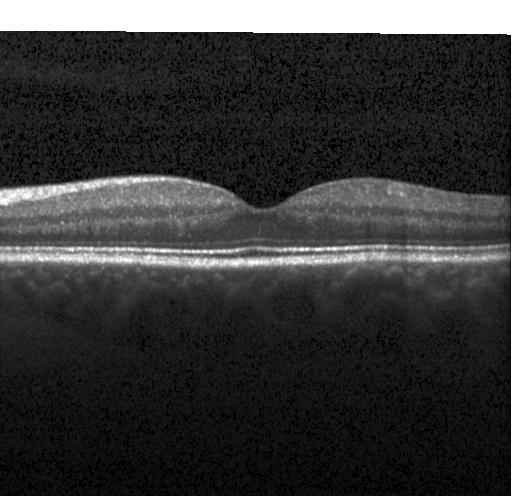

Diagnosis: no evidence of CNV, DME, or drusen.